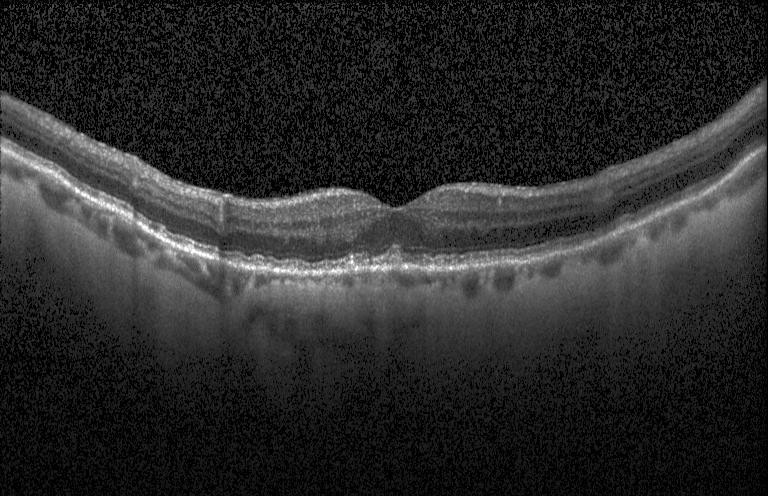

Finding: drusen.